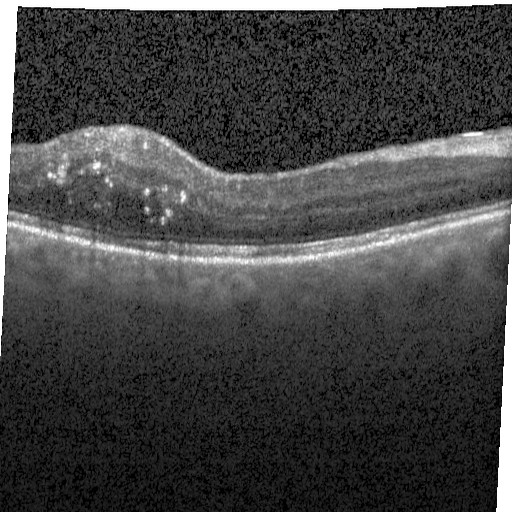

Retinal OCT cross-section · spectral-domain OCT · Heidelberg Spectralis OCT system · centered on the fovea.
Impression: diabetic macular edema (DME).